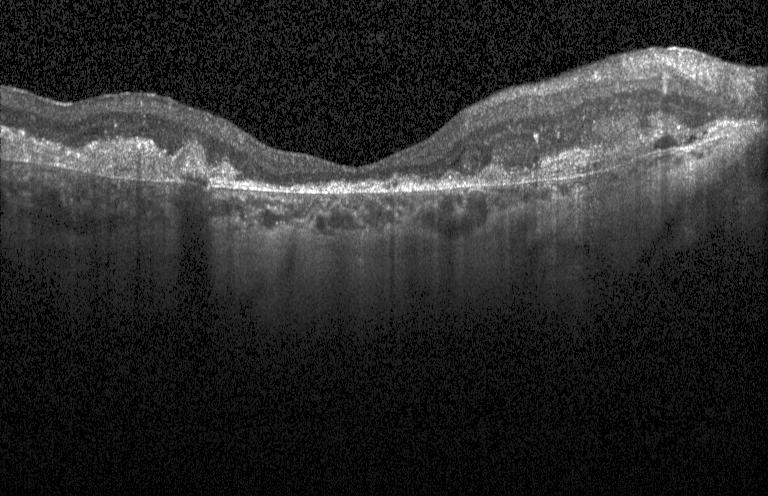 Retinal OCT B-scan
Impression: choroidal neovascularization.